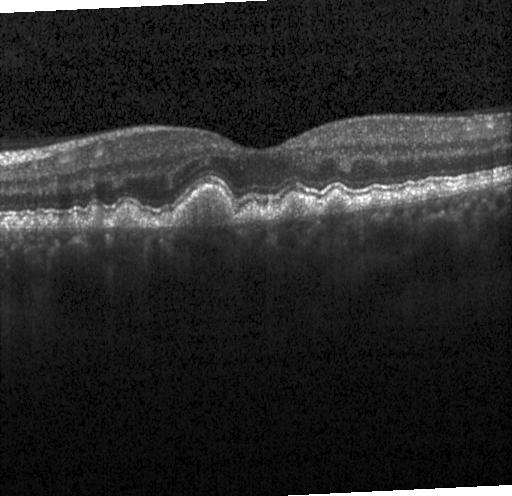

Macular OCT demonstrating drusen.